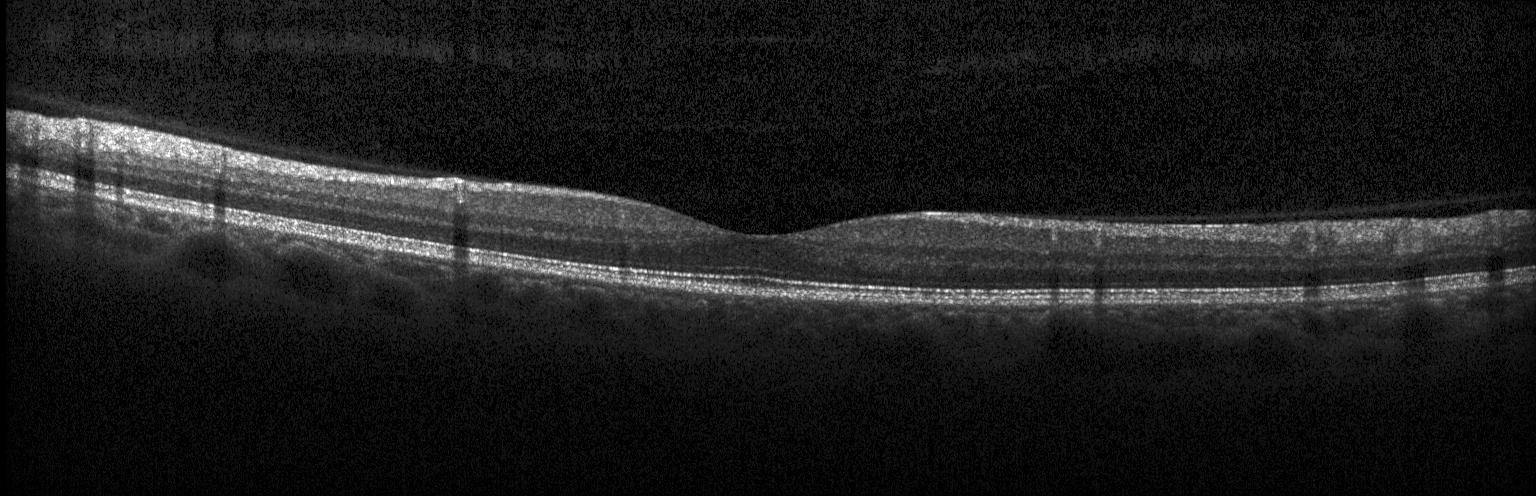

Horizontal scan through the fovea · optical coherence tomography B-scan · instrument: Heidelberg Spectralis
Assessment: no CNV, DME, or drusen.